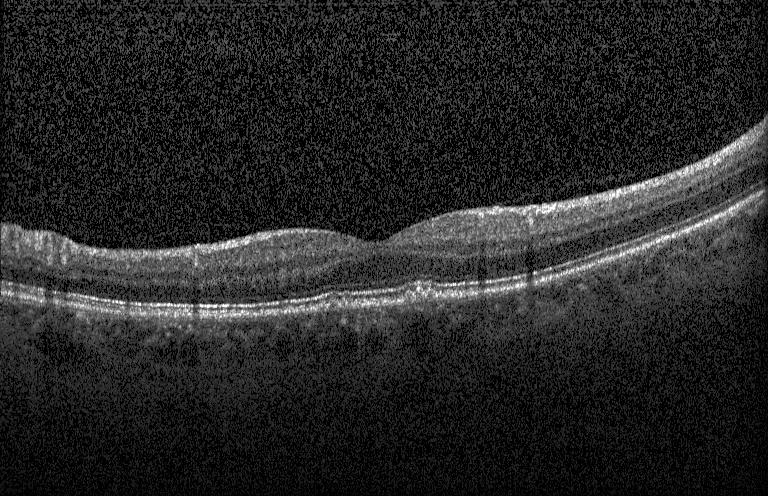 The scan shows multiple drusen.